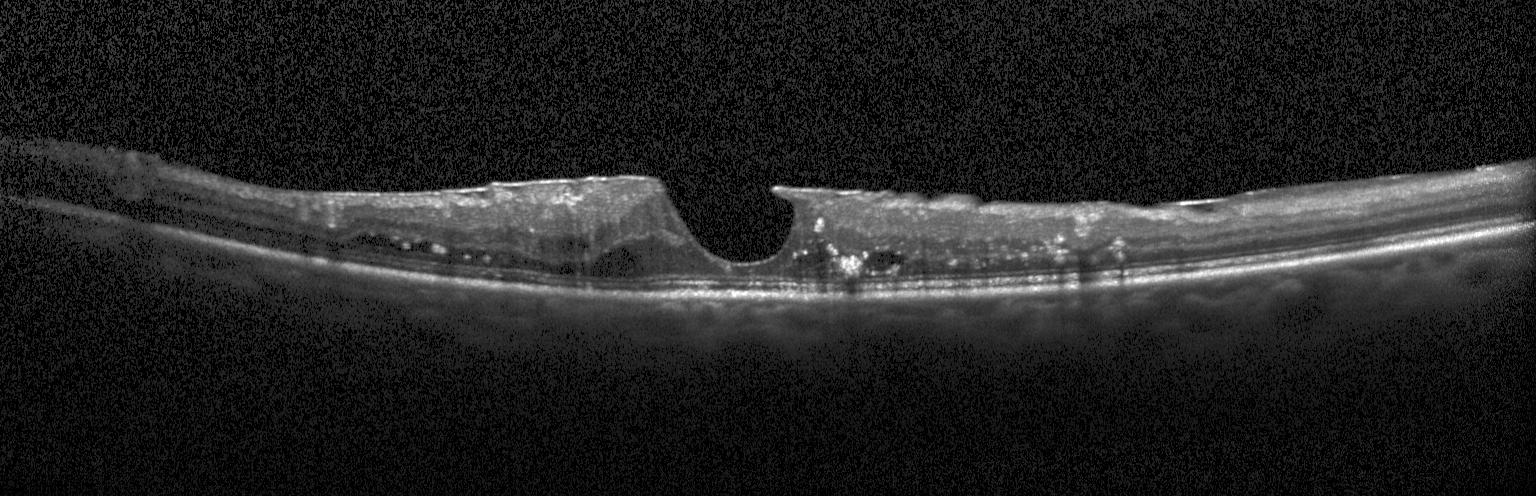
Optical coherence tomography B-scan.
Impression: diabetic macular edema (DME).